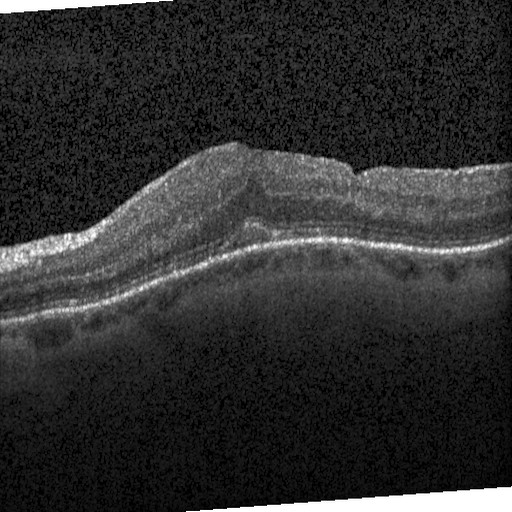 Dx: DME.